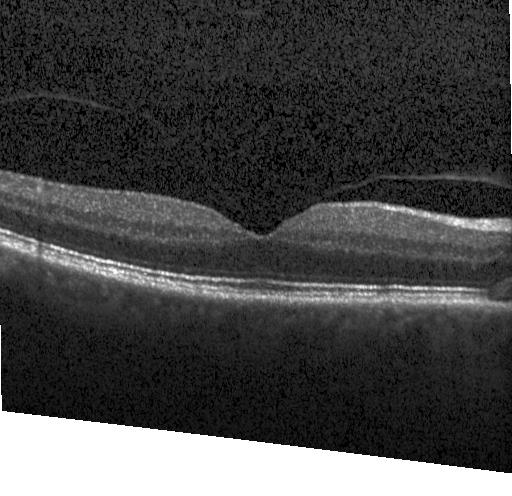

OCT B-scan showing no evidence of choroidal neovascularization, diabetic macular edema, or drusen.